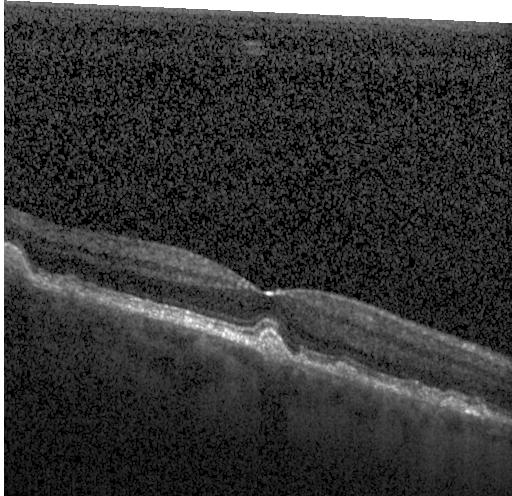

Optical coherence tomography B-scan, Heidelberg Spectralis OCT system, fovea-centered — Drusen.